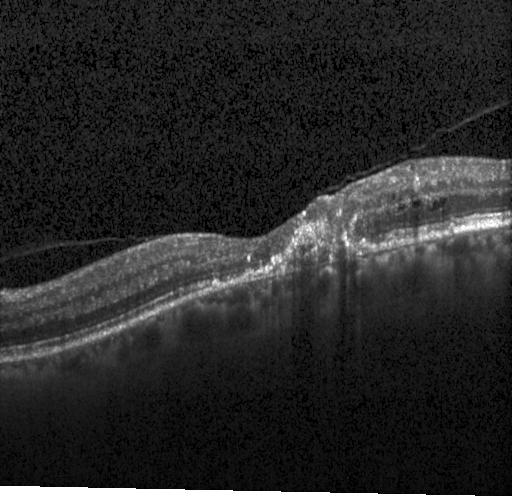 Impression: choroidal neovascularization (CNV).